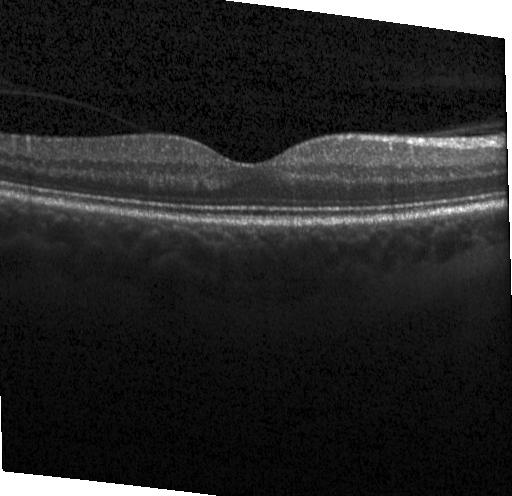

Fovea-centered · acquired on a Heidelberg Spectralis · spectral-domain optical coherence tomography · retinal OCT cross-section. Finding: no CNV, no DME, and no drusen.